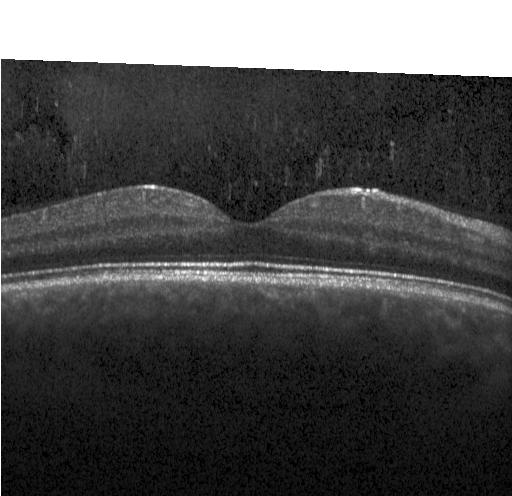 Dx: no choroidal neovascularization, diabetic macular edema, or drusen.